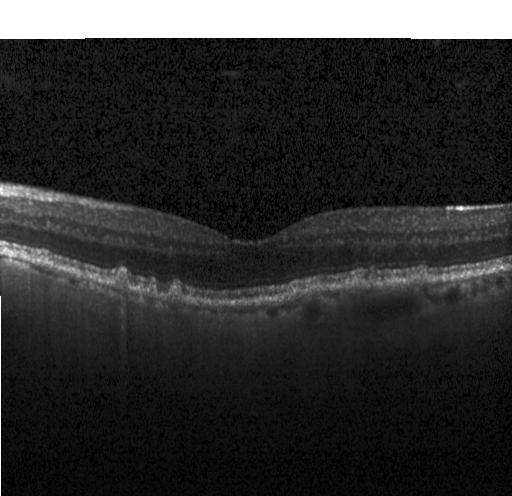

OCT line scan.
The scan shows sub-RPE drusenoid deposits.